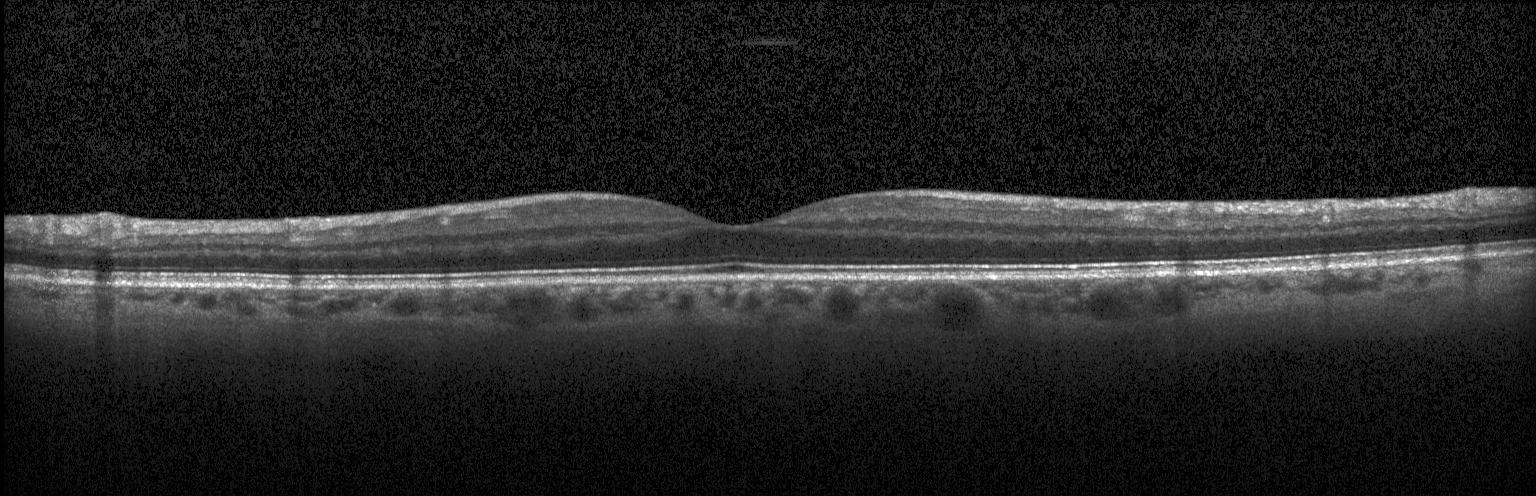
Macular OCT: neither choroidal neovascularization, diabetic macular edema, nor drusen.